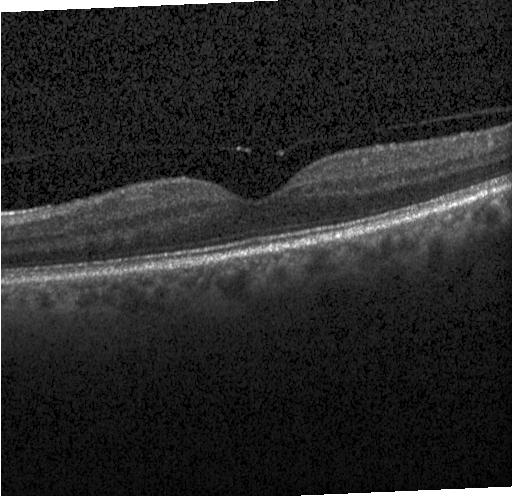

Optical coherence tomography scan — No choroidal neovascularization, no diabetic macular edema, and no drusen.